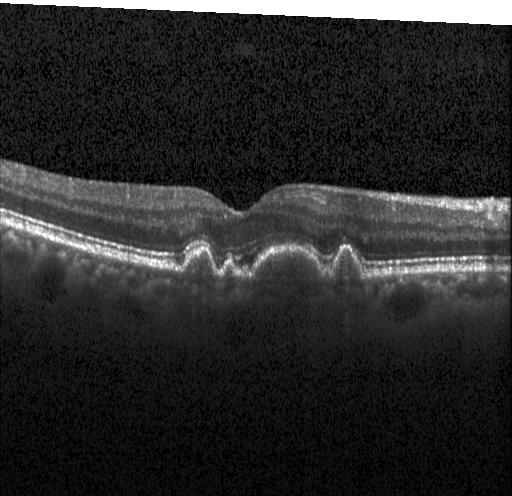
OCT B-scan.
Impression: drusen.